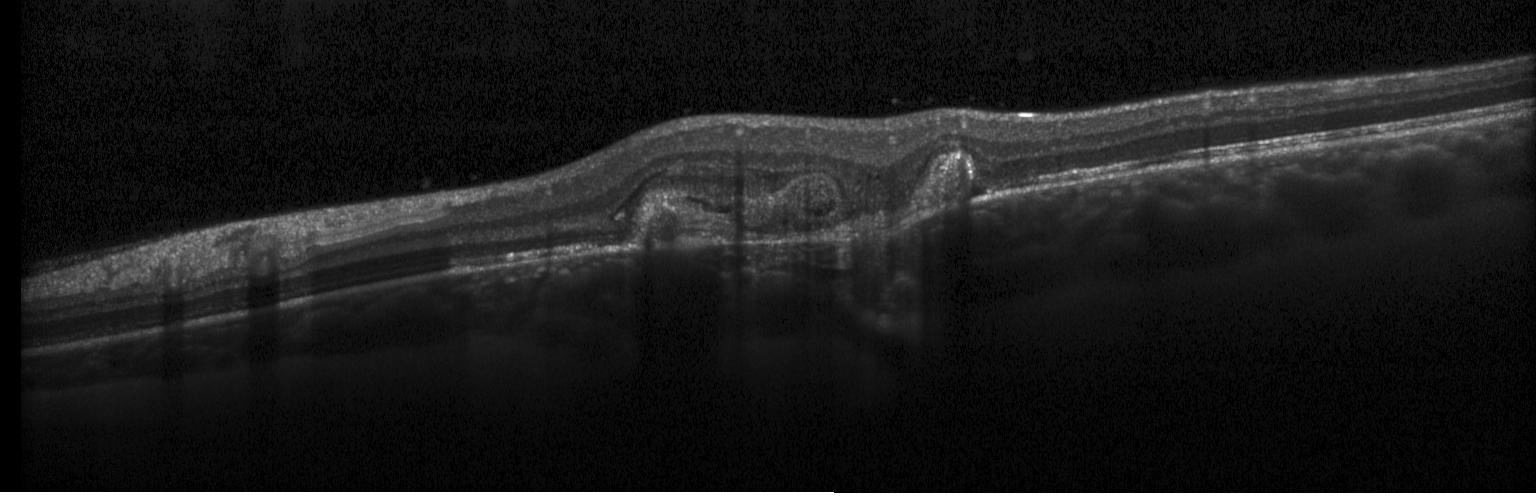
Retinal OCT B-scan — Assessment: a choroidal neovascular membrane.